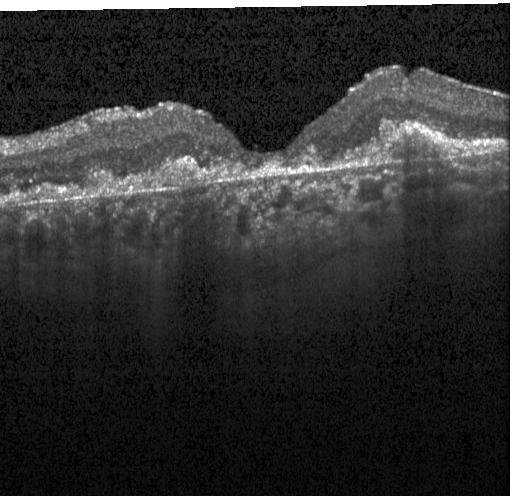
OCT line scan. SD-OCT. Macular scan. This B-scan demonstrates CNV.